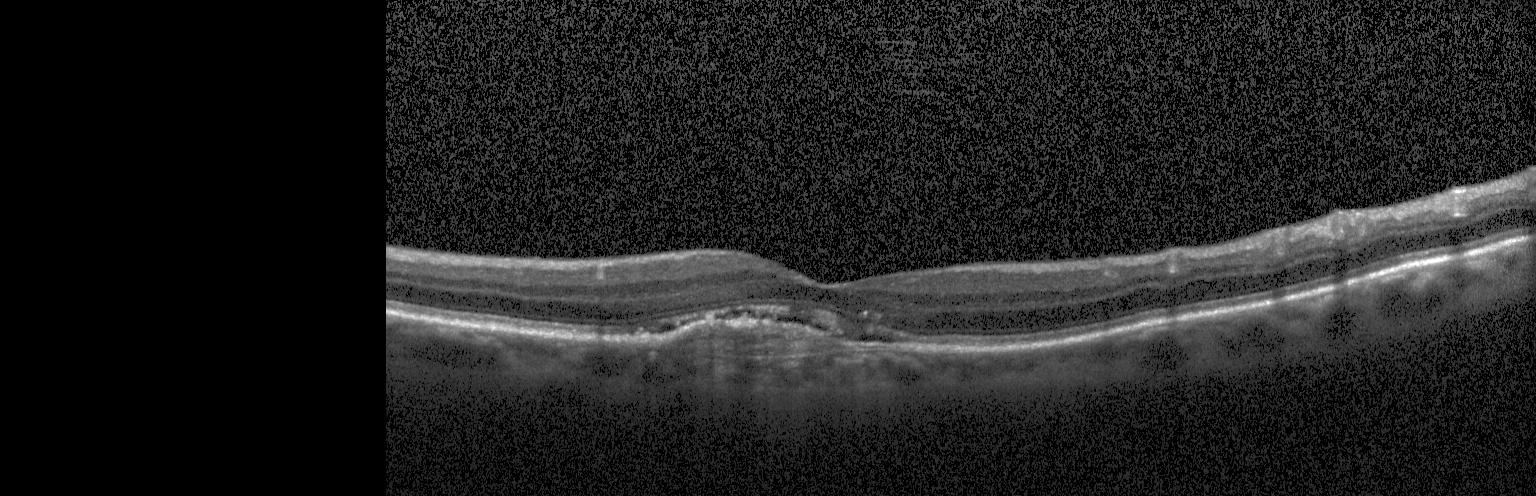

OCT finding: a choroidal neovascular membrane.